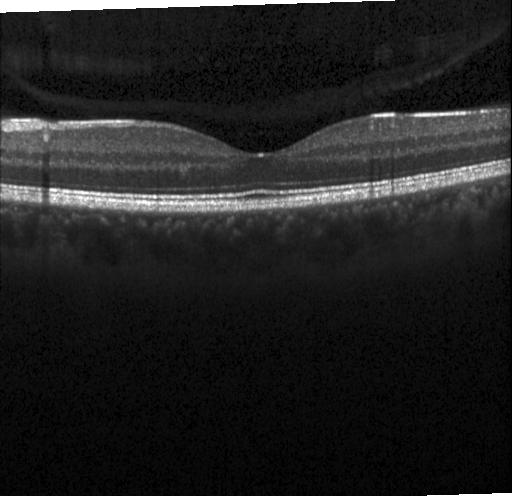 OCT finding: no choroidal neovascularization, no diabetic macular edema, and no drusen.